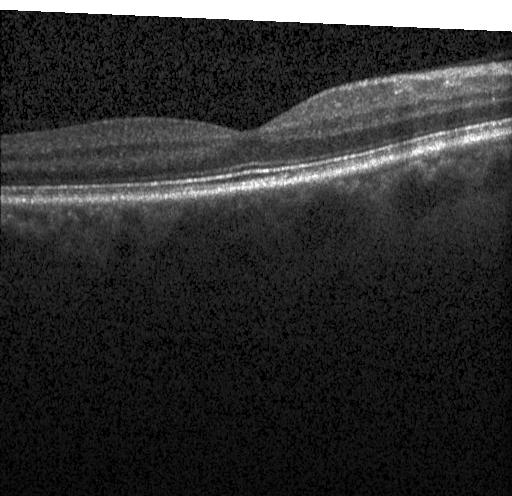
Impression: no evidence of choroidal neovascularization, diabetic macular edema, or drusen.